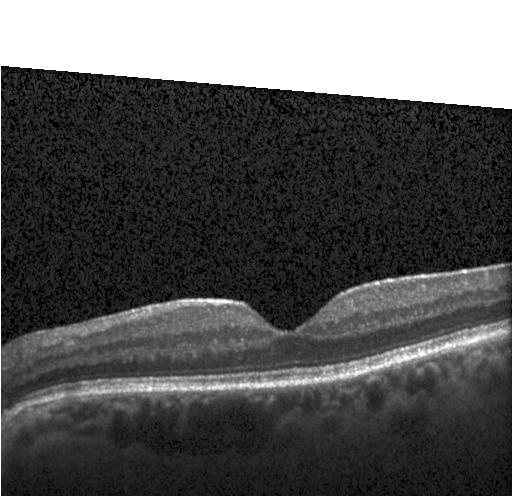
No CNV, no DME, and no drusen.